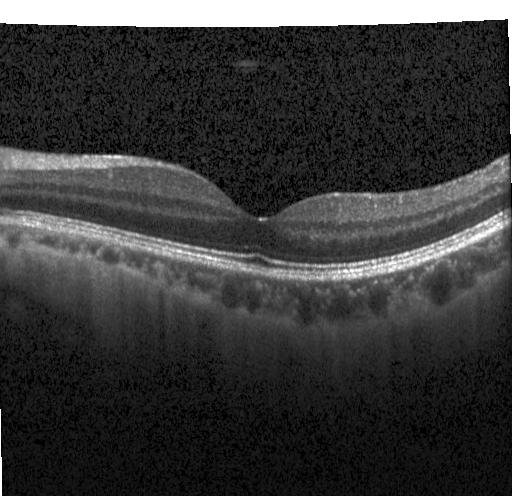
Retinal OCT B-scan; horizontal scan through the fovea; Heidelberg Spectralis.
Finding: no choroidal neovascularization, no diabetic macular edema, and no drusen.